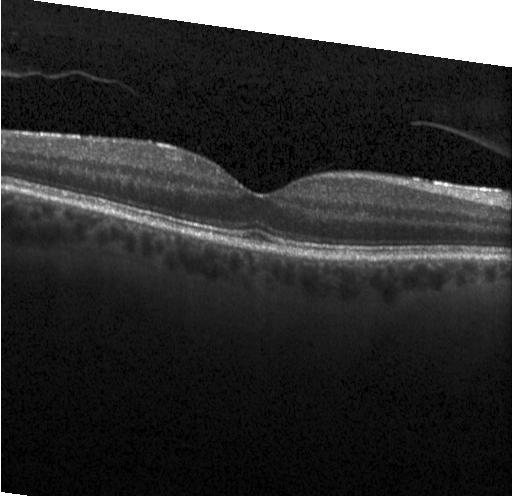

Heidelberg Spectralis OCT system. Retinal OCT B-scan. SD-OCT
No evidence of CNV, DME, or drusen.